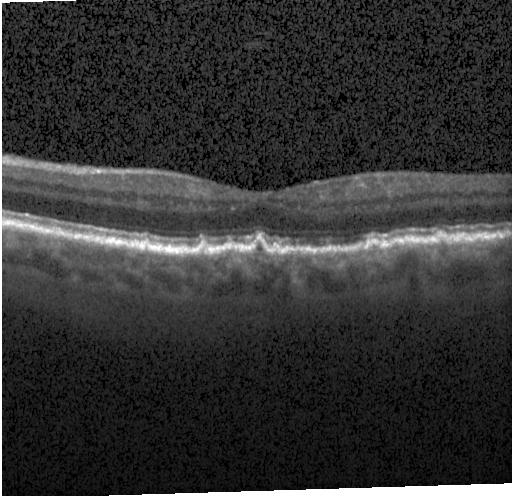
Dx: sub-RPE drusenoid deposits.